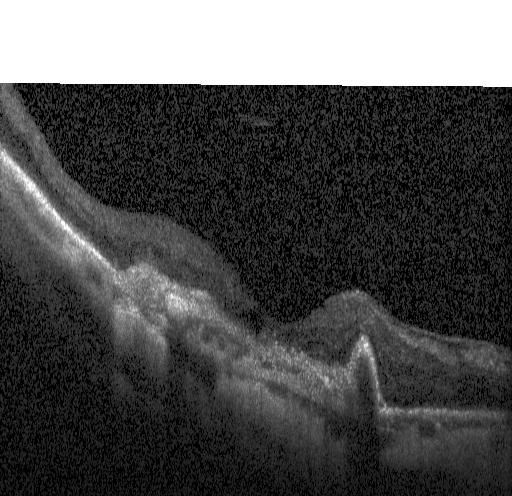
Dx: choroidal neovascularization (CNV).